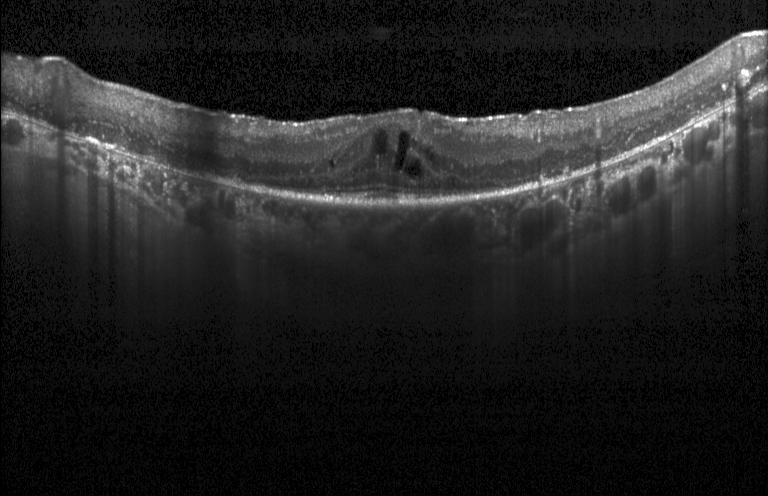

Macular OCT: diabetic macular edema.